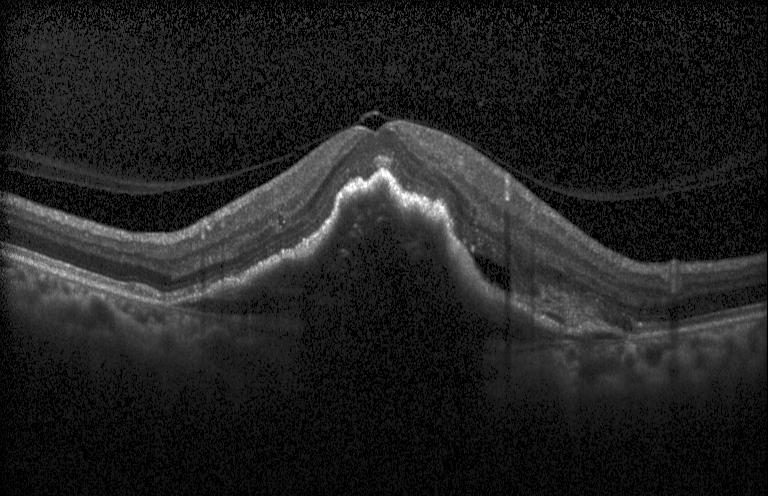

The scan shows CNV.